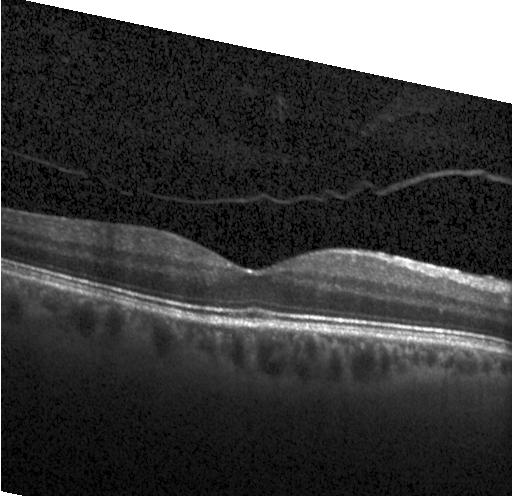

Assessment: neither CNV, DME, nor drusen.